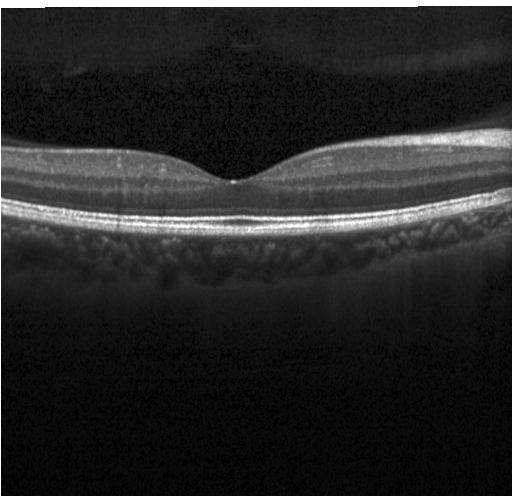
Optical coherence tomography scan — Diagnosis: no CNV, no DME, and no drusen.